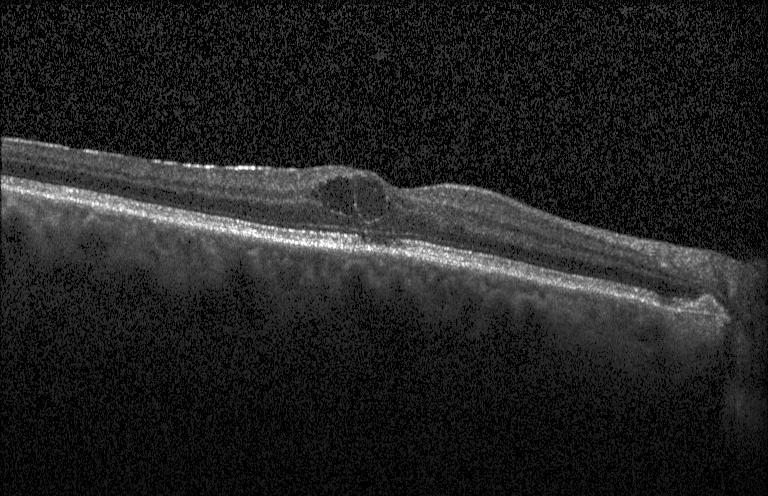 SD-OCT. Horizontal scan through the fovea. Instrument: Heidelberg Spectralis. Optical coherence tomography B-scan.
The scan shows DME.